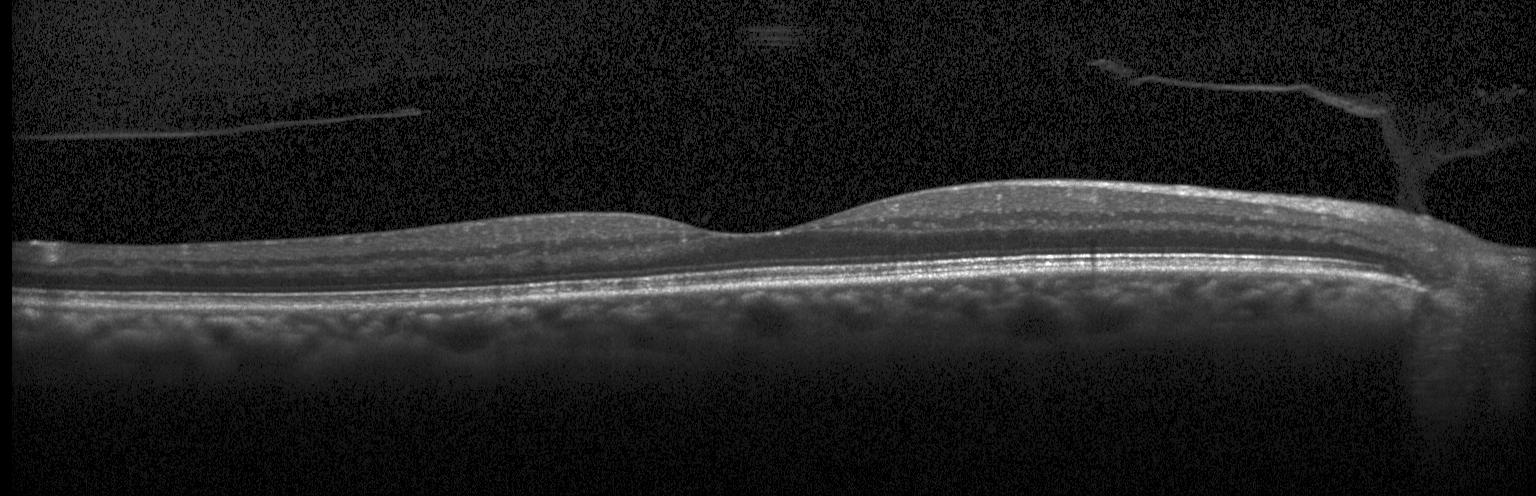
OCT B-scan showing no choroidal neovascularization, diabetic macular edema, or drusen.